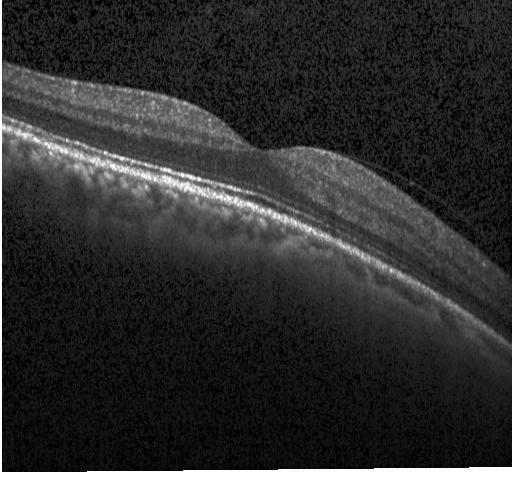 OCT B-scan showing neither choroidal neovascularization, diabetic macular edema, nor drusen.